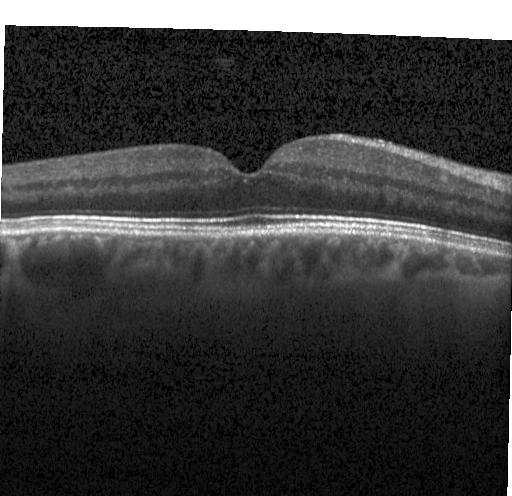 Impression: no choroidal neovascularization, no diabetic macular edema, and no drusen.